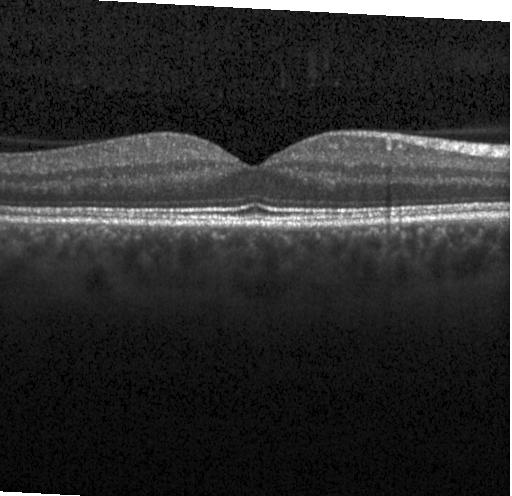
Retinal OCT cross-section. No evidence of choroidal neovascularization, diabetic macular edema, or drusen.